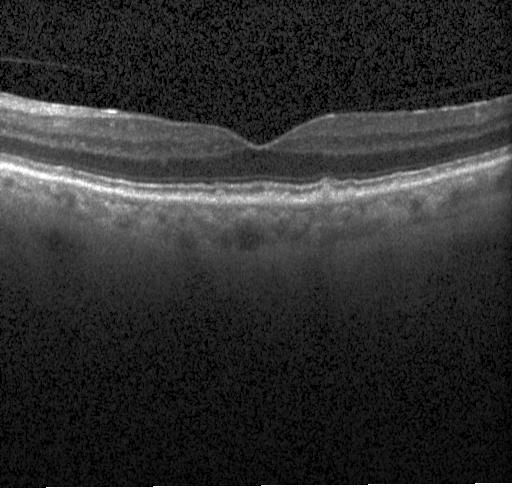 Centered on the fovea · OCT B-scan · spectral-domain optical coherence tomography — Finding: multiple drusen.